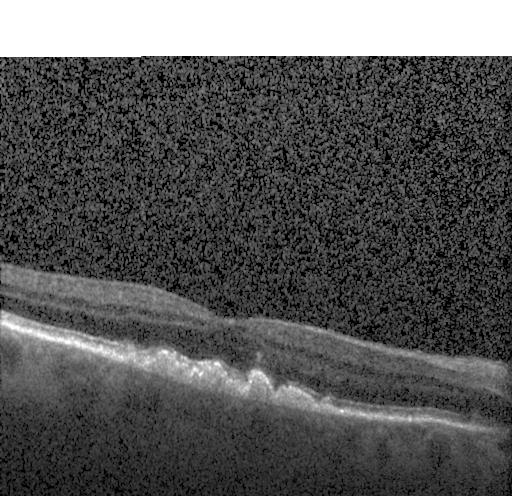 Retinal OCT cross-section
Diagnosis: drusen.